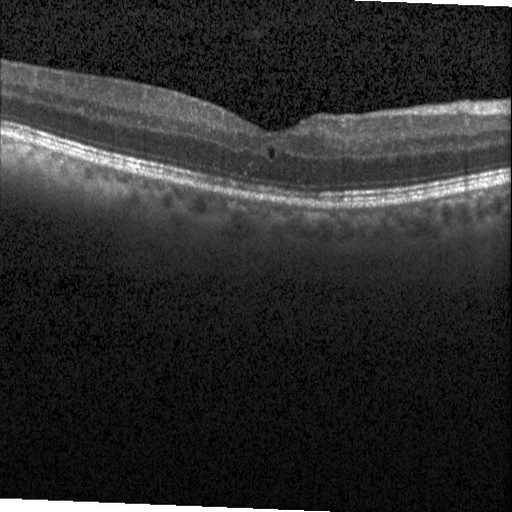

Retinal OCT B-scan; instrument: Heidelberg Spectralis — Finding: DME.